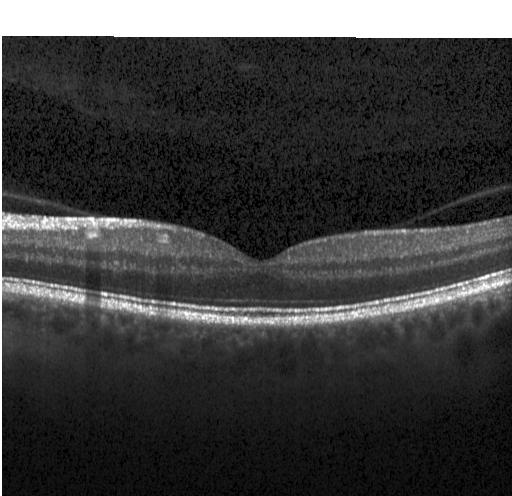
Impression: no evidence of CNV, DME, or drusen.